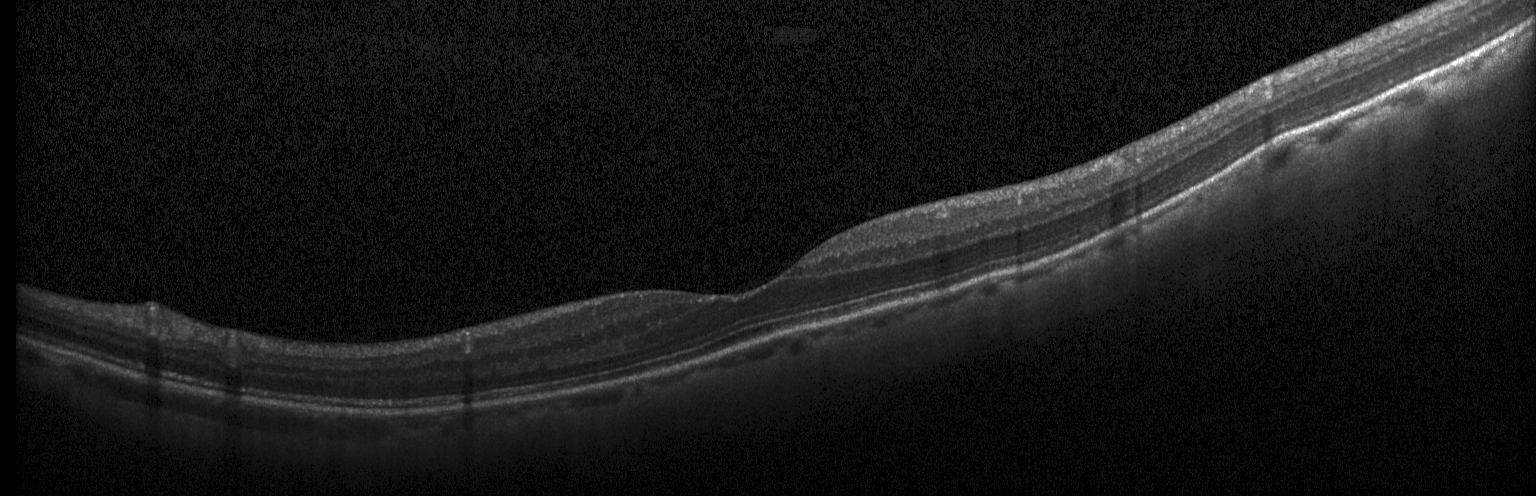
Optical coherence tomography B-scan.
OCT finding: no evidence of CNV, DME, or drusen.